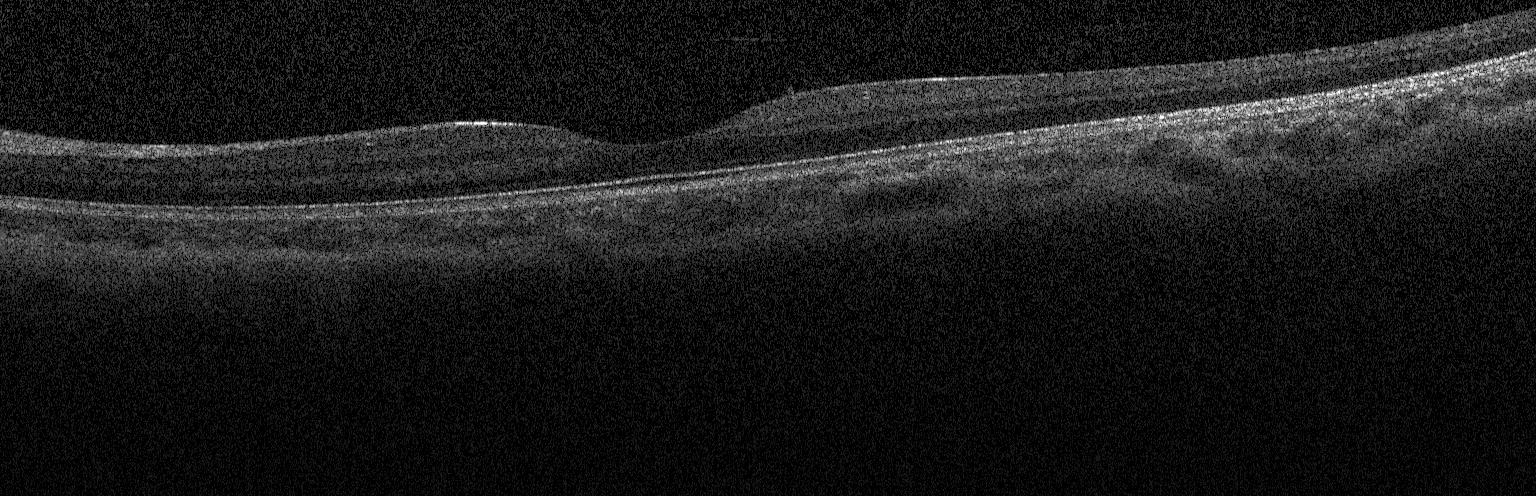

Heidelberg Spectralis OCT system; optical coherence tomography scan — Finding: no evidence of choroidal neovascularization, diabetic macular edema, or drusen.